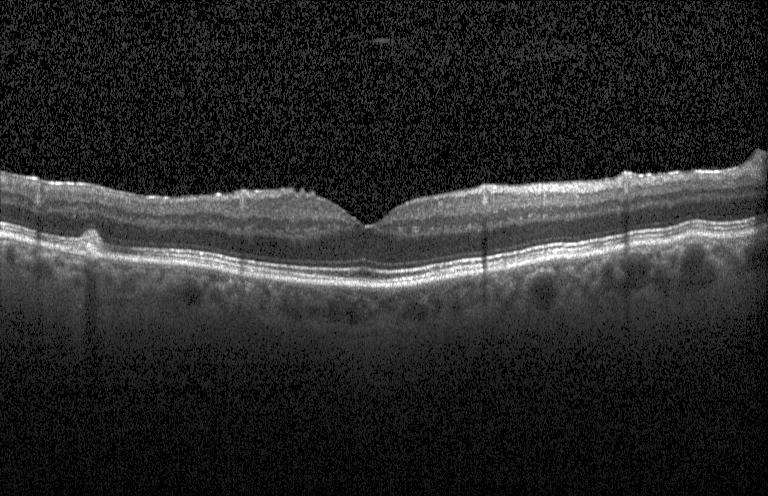
Dx: drusen.